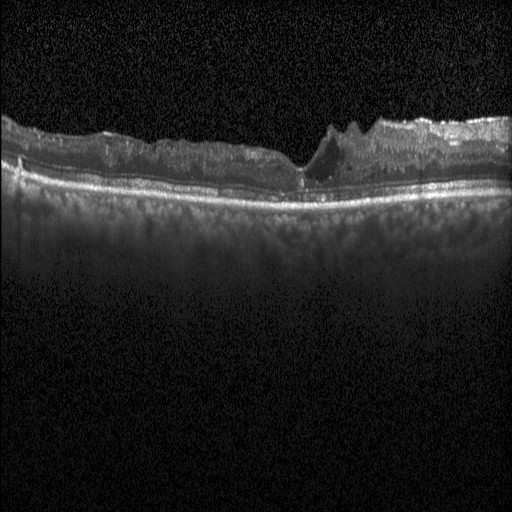

Optical coherence tomography B-scan; centered on the fovea; Heidelberg Spectralis OCT system — Impression: diabetic macular edema.